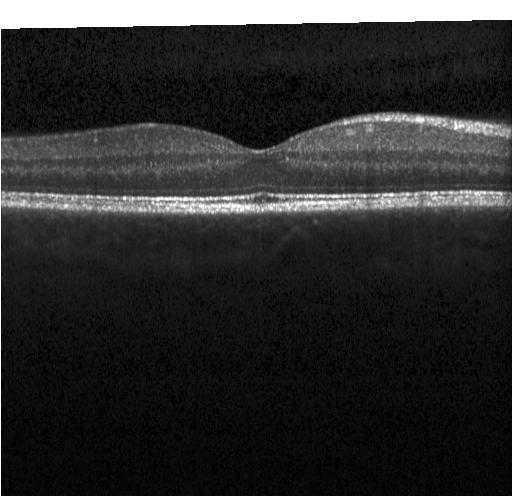

Impression: no evidence of choroidal neovascularization, diabetic macular edema, or drusen.